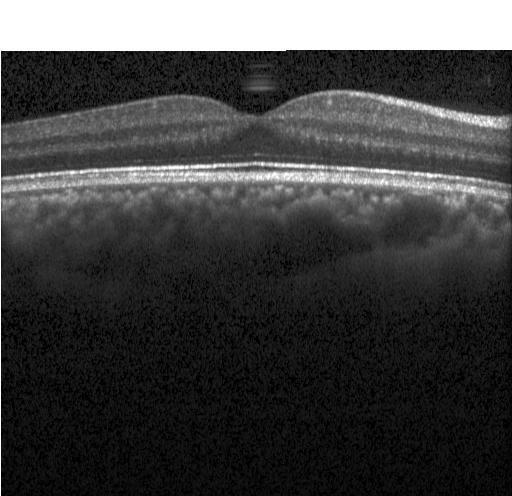 Macular OCT: no CNV, DME, or drusen.